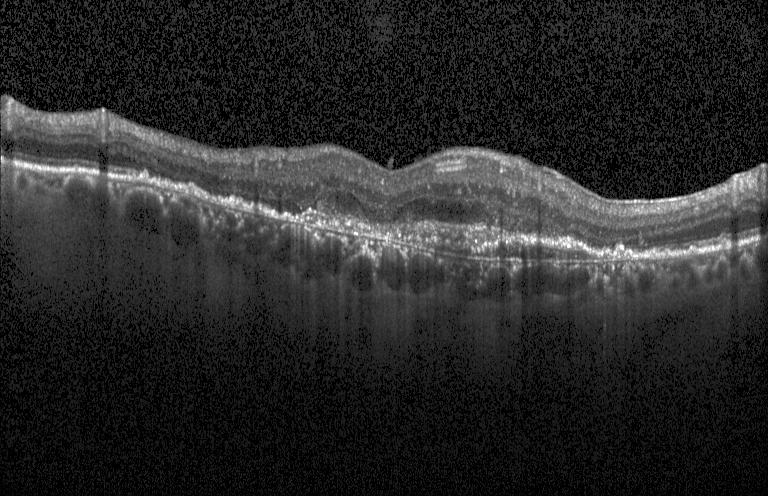

Impression: a choroidal neovascular membrane.